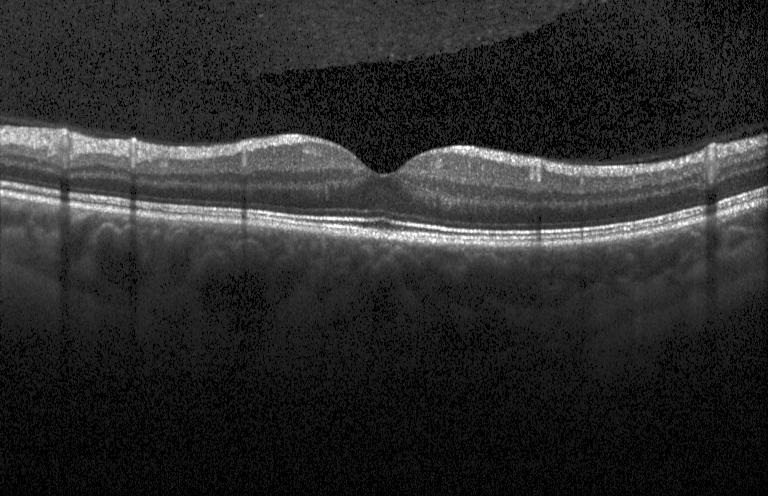
Macular OCT: no choroidal neovascularization, no diabetic macular edema, and no drusen.